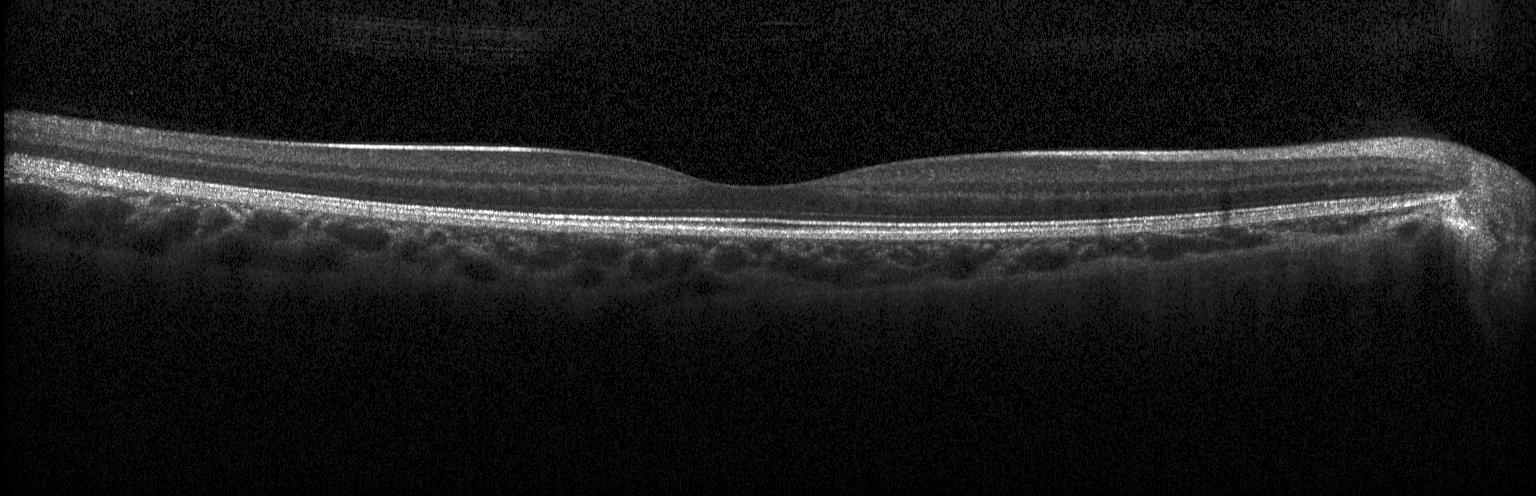

Diagnosis: neither choroidal neovascularization, diabetic macular edema, nor drusen.